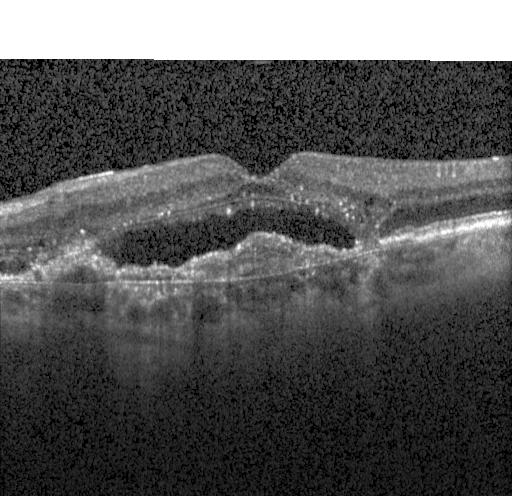 Horizontal scan through the fovea. OCT B-scan. Spectral-domain OCT.
Macular OCT: choroidal neovascularization.